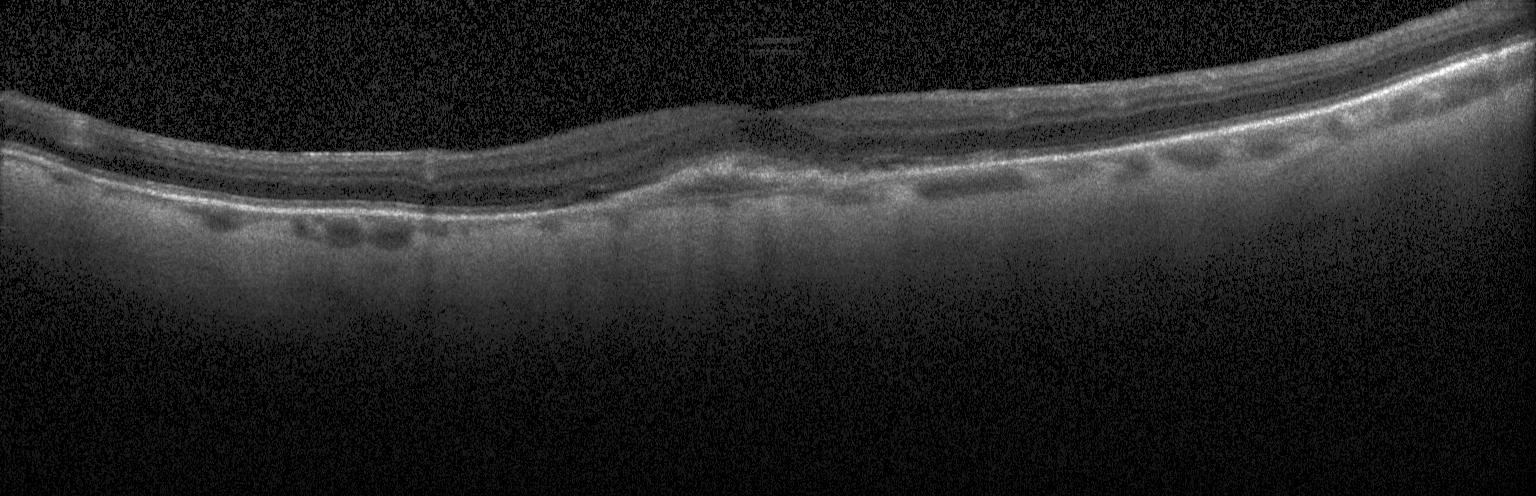

Retinal OCT cross-section. Macular OCT: a choroidal neovascular membrane.